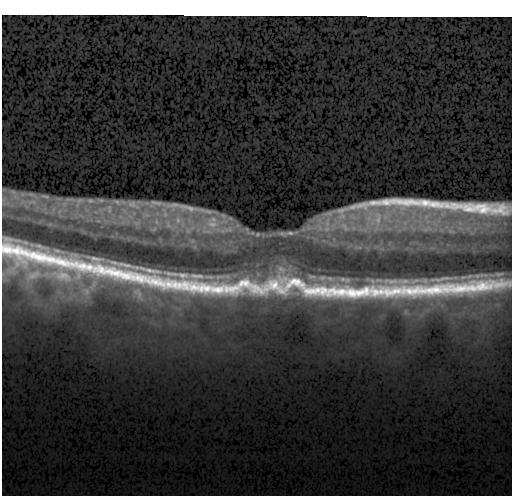 Heidelberg Spectralis OCT system, retinal OCT B-scan, SD-OCT, through the macula. Diagnosis: multiple drusen.